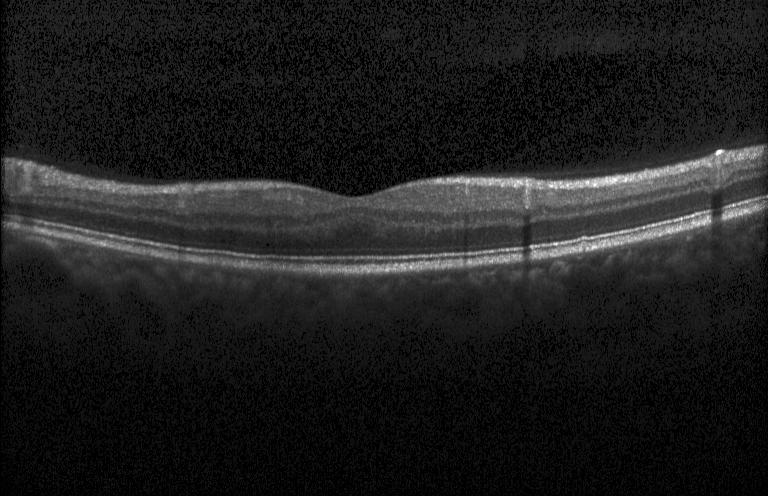 Diagnosis: no choroidal neovascularization, no diabetic macular edema, and no drusen.